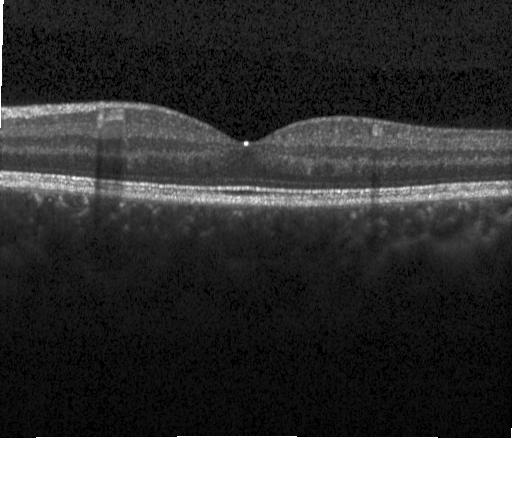
OCT B-scan showing neither choroidal neovascularization, diabetic macular edema, nor drusen.